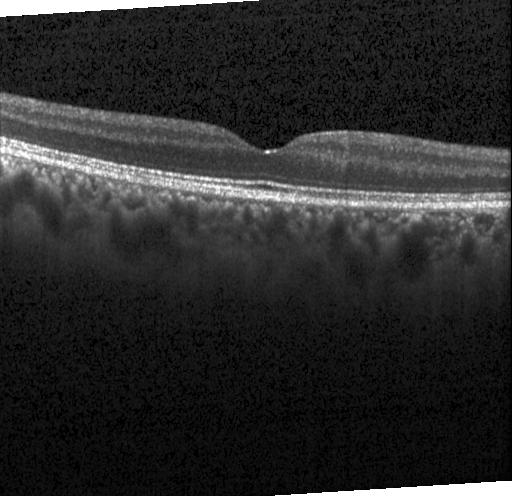
Assessment: neither CNV, DME, nor drusen.